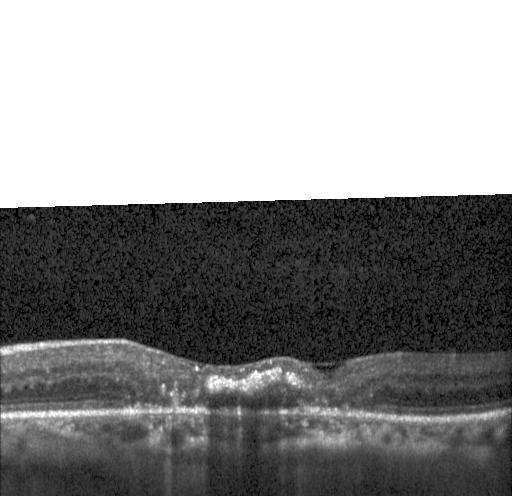
Macular OCT demonstrating choroidal neovascularization.